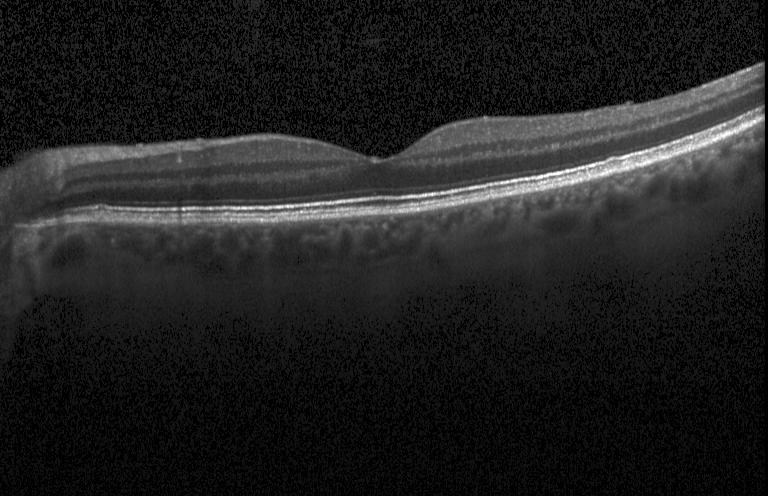 Macular OCT demonstrating neither CNV, DME, nor drusen.